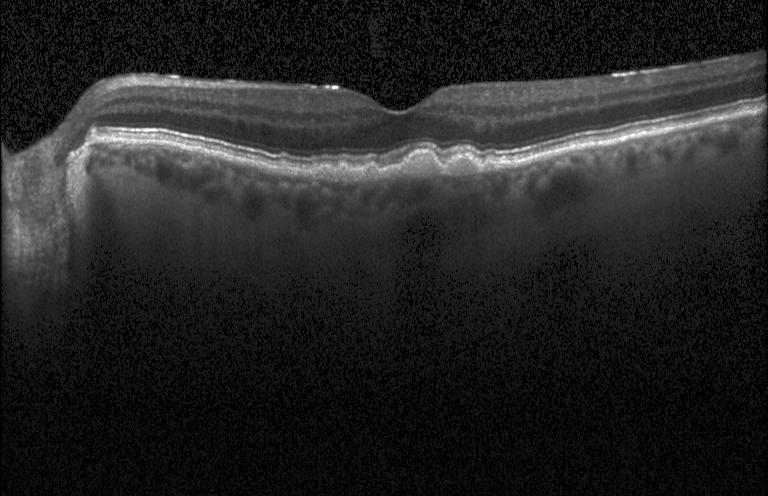
Spectral-domain OCT. Retinal OCT cross-section. Heidelberg Spectralis — Assessment: multiple drusen.